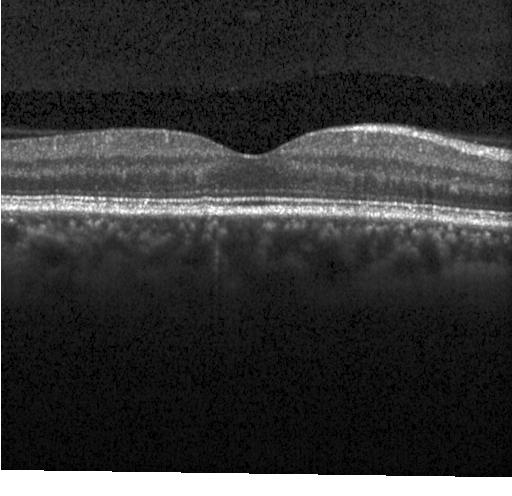
Centered on the fovea. Retinal OCT cross-section. Spectral-domain OCT.
Finding: no CNV, no DME, and no drusen.